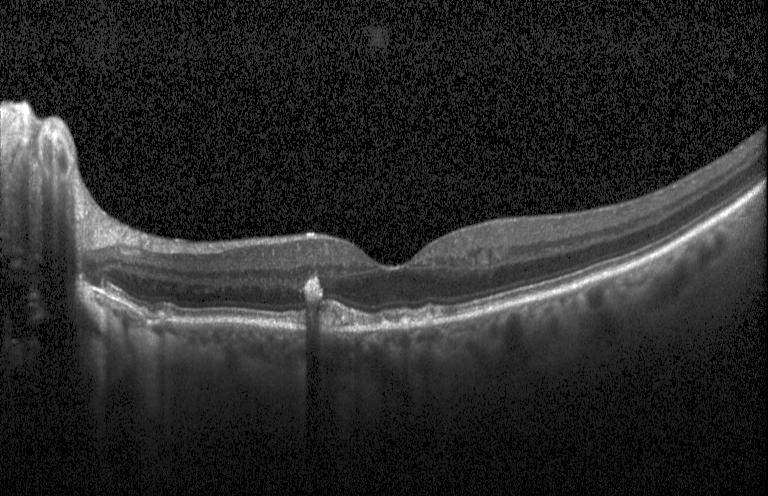
Macular scan. Retinal OCT cross-section. Impression: multiple drusen.